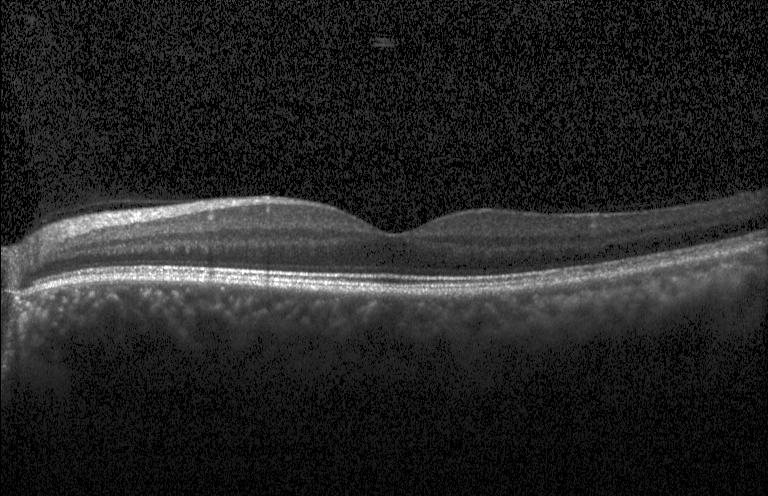

Retinal OCT B-scan
Finding: no choroidal neovascularization, diabetic macular edema, or drusen.